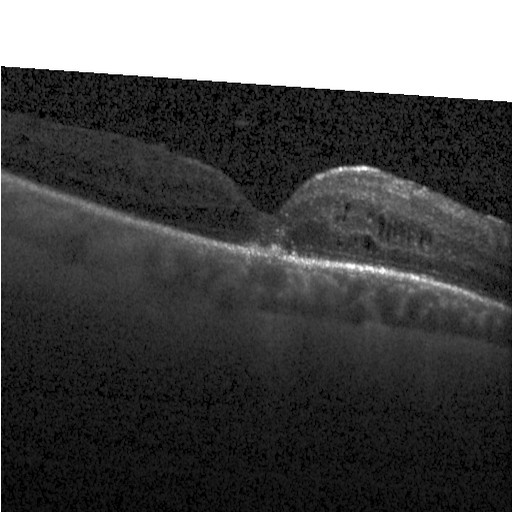
Macular OCT: diabetic macular edema.